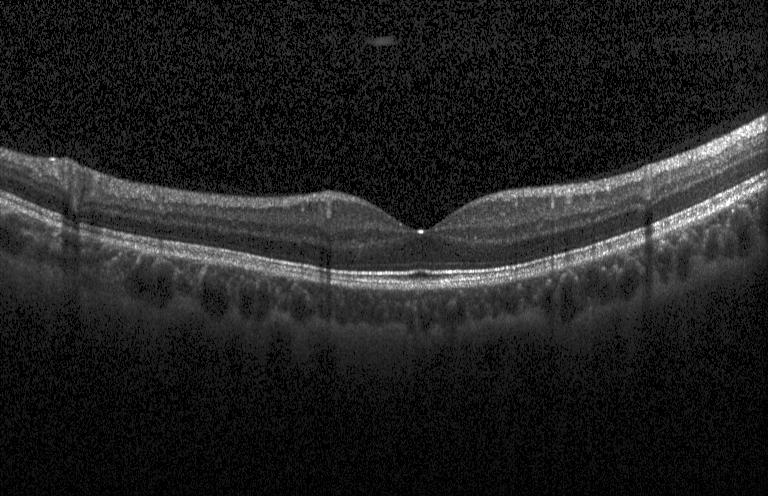

Horizontal scan through the fovea, optical coherence tomography scan, Heidelberg Spectralis, spectral-domain OCT
No CNV, no DME, and no drusen.